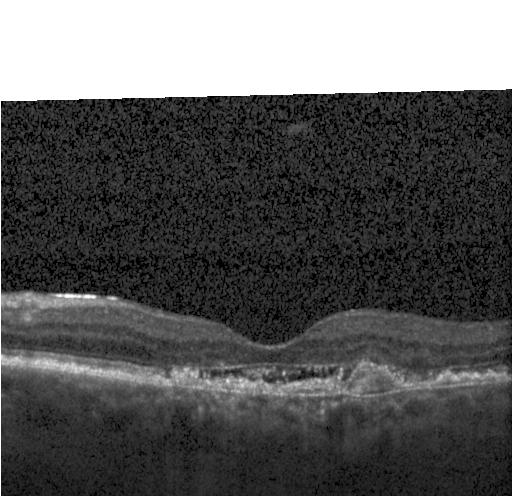 Fovea-centered, acquired on a Heidelberg Spectralis, optical coherence tomography scan, spectral-domain OCT.
Assessment: choroidal neovascularization (CNV).